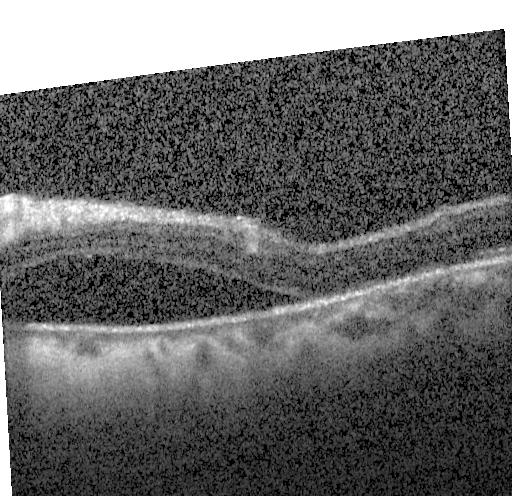

OCT scan showing choroidal neovascularization.